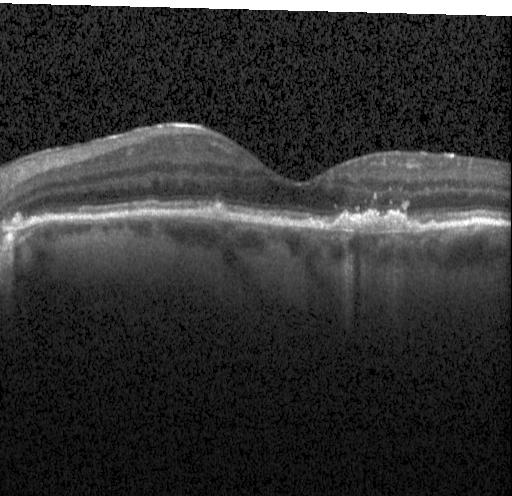 Optical coherence tomography B-scan
Assessment: sub-RPE drusenoid deposits.